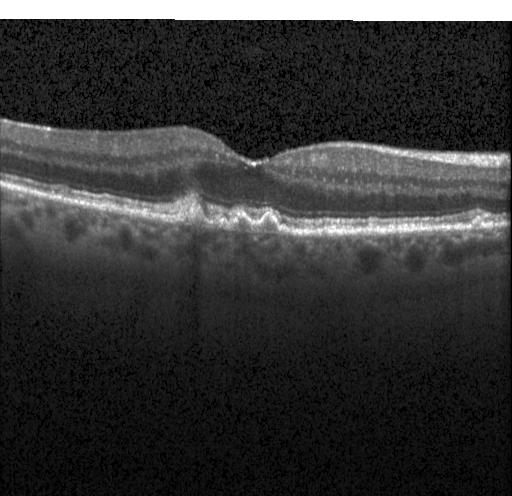 SD-OCT, OCT B-scan.
Sub-RPE drusenoid deposits.